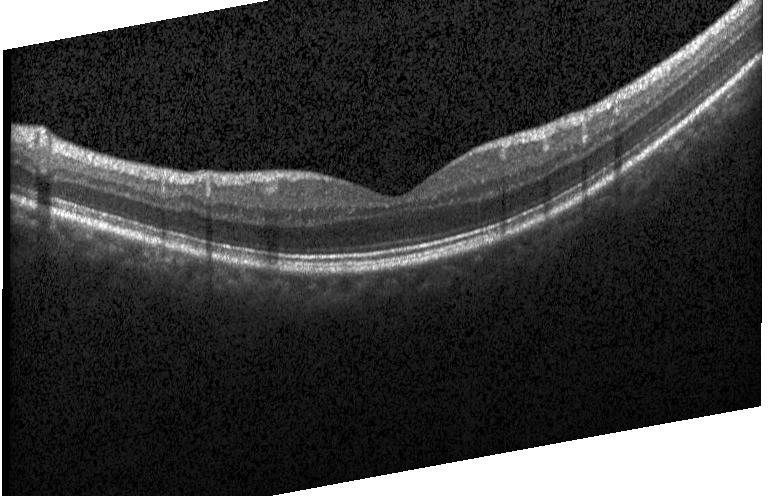 OCT B-scan, spectral-domain optical coherence tomography.
Finding: no evidence of choroidal neovascularization, diabetic macular edema, or drusen.